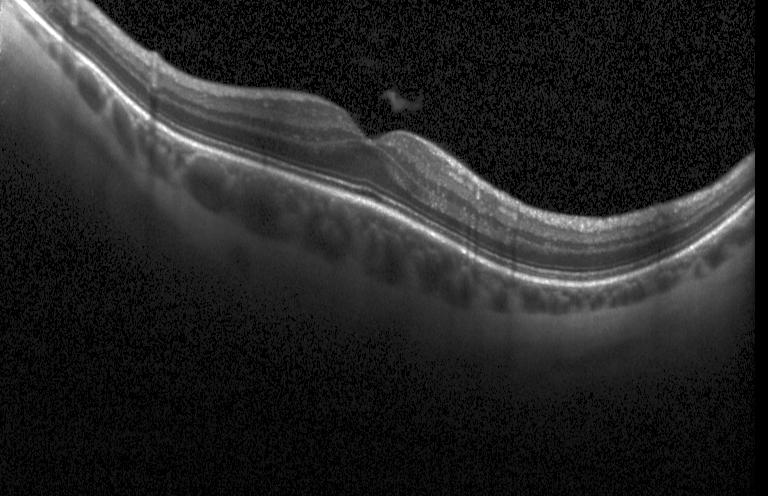 Finding: no evidence of choroidal neovascularization, diabetic macular edema, or drusen.